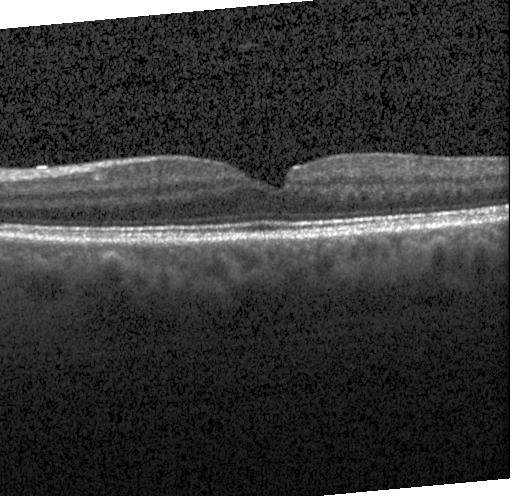

Spectral-domain OCT · acquired on a Heidelberg Spectralis · optical coherence tomography scan.
Finding: no choroidal neovascularization, no diabetic macular edema, and no drusen.